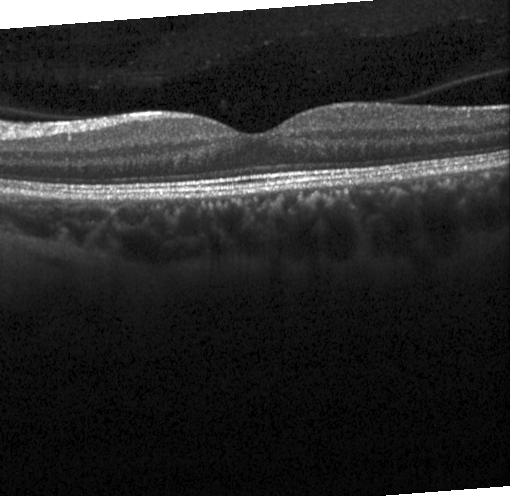

Acquired on a Heidelberg Spectralis · horizontal scan through the fovea · optical coherence tomography scan · spectral-domain optical coherence tomography — Diagnosis: no evidence of CNV, DME, or drusen.